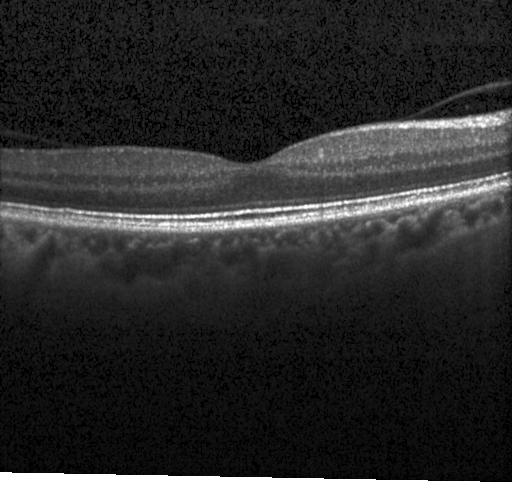

Retinal OCT cross-section; Heidelberg Spectralis OCT system.
Impression: neither CNV, DME, nor drusen.